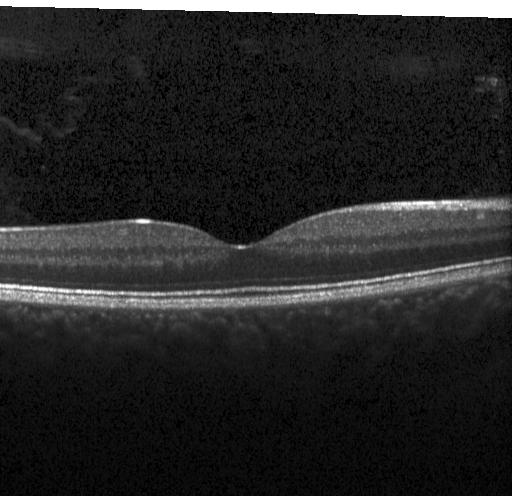
Through the macula. Heidelberg Spectralis. Optical coherence tomography scan — Diagnosis: neither choroidal neovascularization, diabetic macular edema, nor drusen.